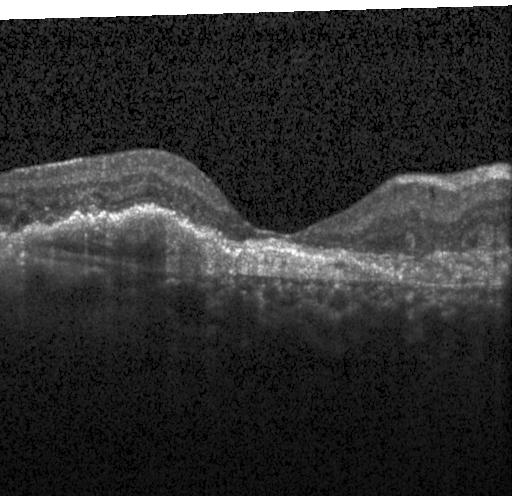

Spectral-domain optical coherence tomography; optical coherence tomography B-scan; macular scan
Macular OCT: choroidal neovascularization.